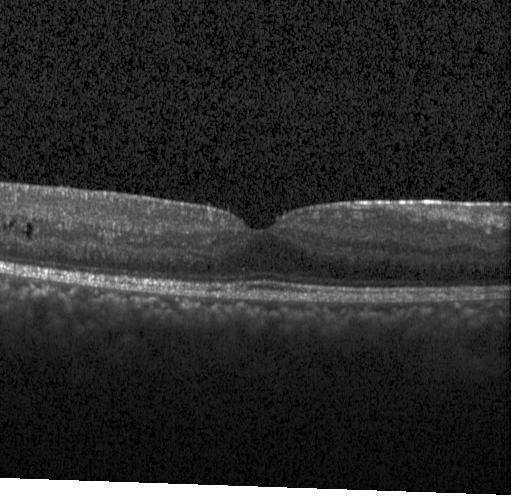
Centered on the fovea · Heidelberg Spectralis OCT system · retinal OCT cross-section · SD-OCT.
The scan shows DME.